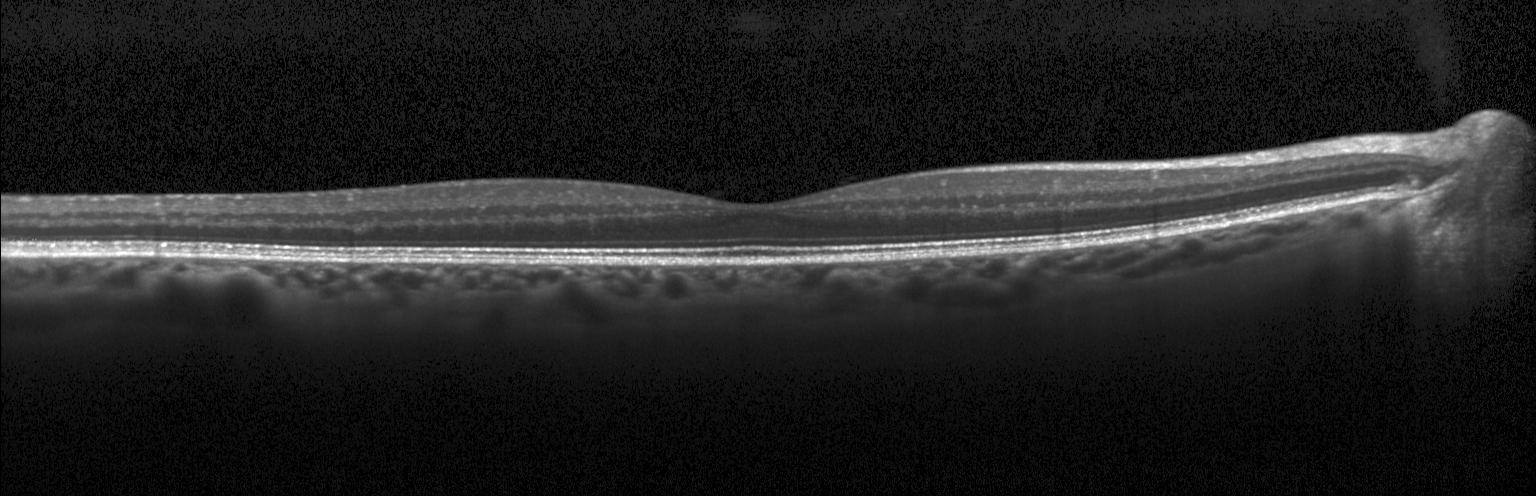 Fovea-centered. Optical coherence tomography B-scan
The scan shows no choroidal neovascularization, no diabetic macular edema, and no drusen.